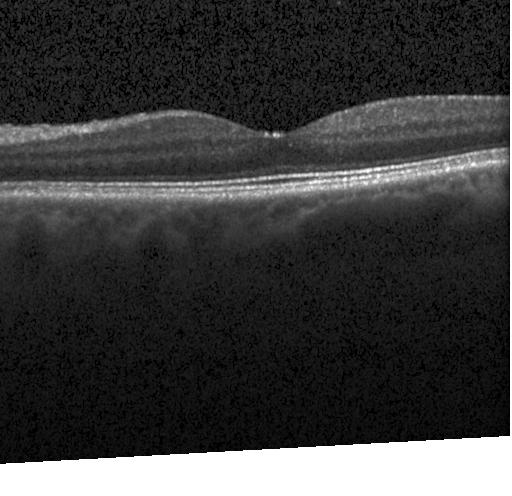

Acquired on a Heidelberg Spectralis; retinal OCT cross-section; fovea-centered; SD-OCT.
OCT finding: no CNV, no DME, and no drusen.